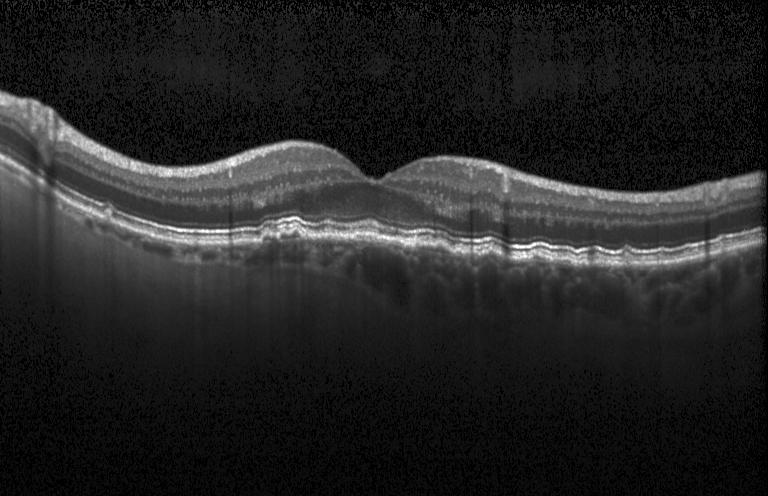

Spectral-domain OCT. OCT line scan.
The scan shows multiple drusen.